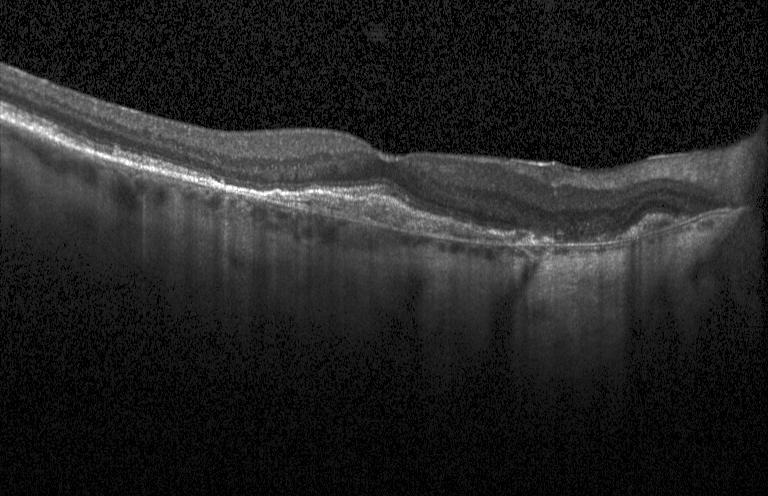
The scan shows a choroidal neovascular membrane.